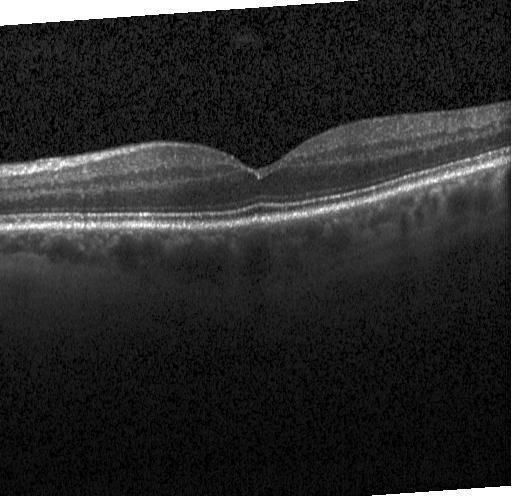 Diagnosis: neither CNV, DME, nor drusen.